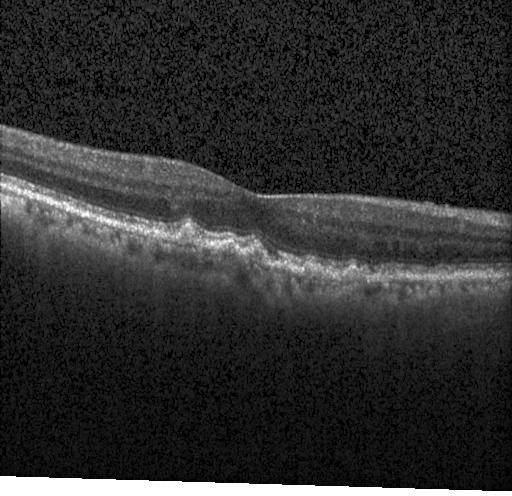

The scan shows multiple drusen.